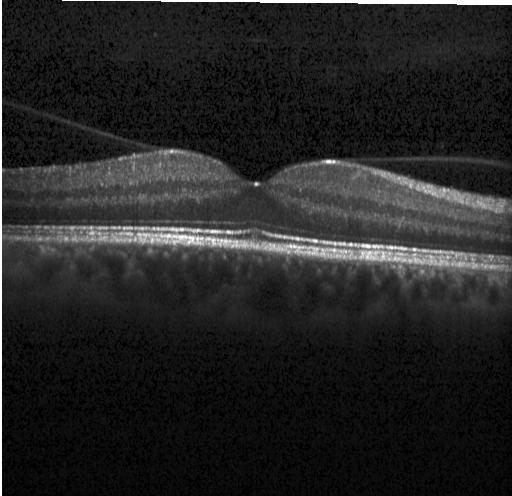
OCT B-scan. No CNV, no DME, and no drusen.